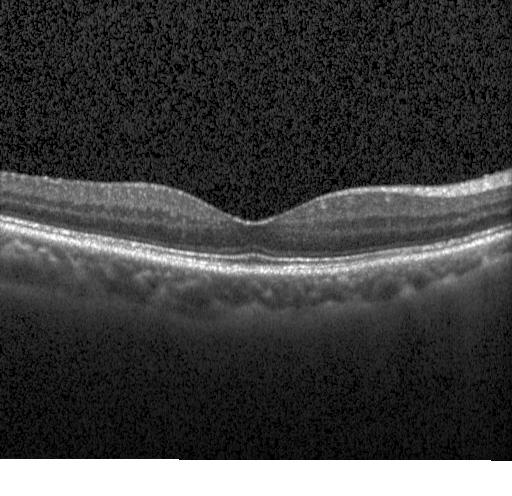 Instrument: Heidelberg Spectralis · retinal OCT B-scan · spectral-domain OCT — Finding: no evidence of choroidal neovascularization, diabetic macular edema, or drusen.